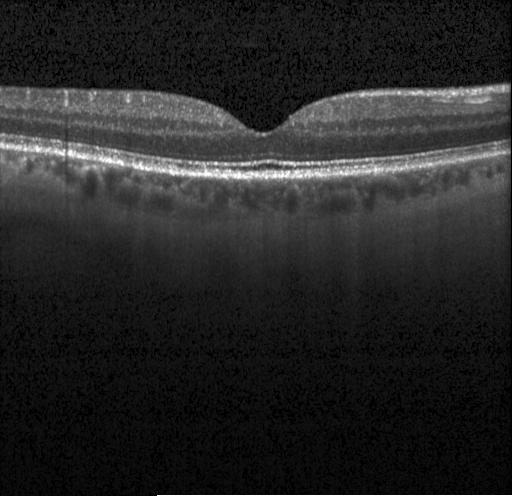
Impression: no CNV, DME, or drusen.